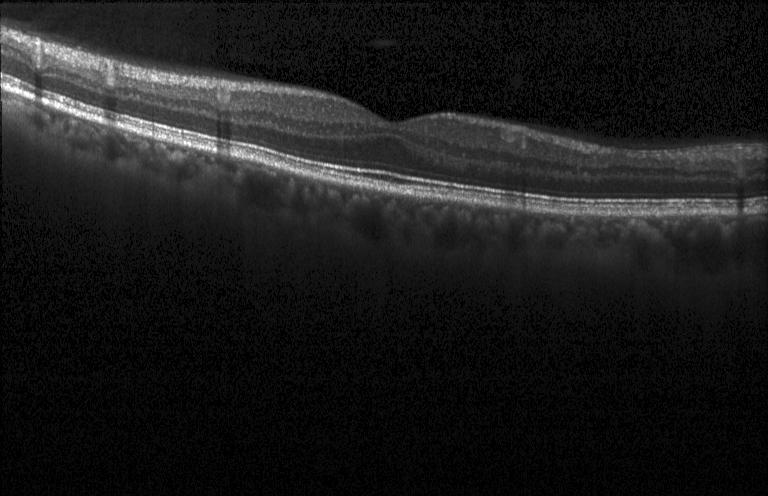 Instrument: Heidelberg Spectralis, optical coherence tomography B-scan, spectral-domain optical coherence tomography
No evidence of choroidal neovascularization, diabetic macular edema, or drusen.